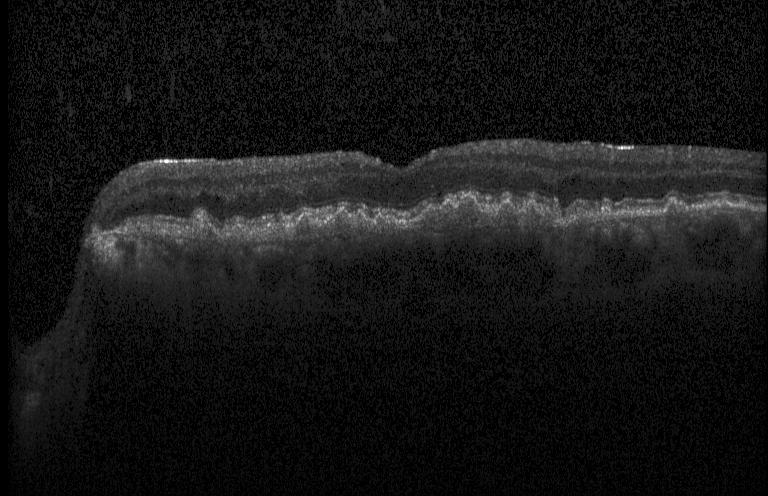
OCT line scan. Macular OCT: a choroidal neovascular membrane.